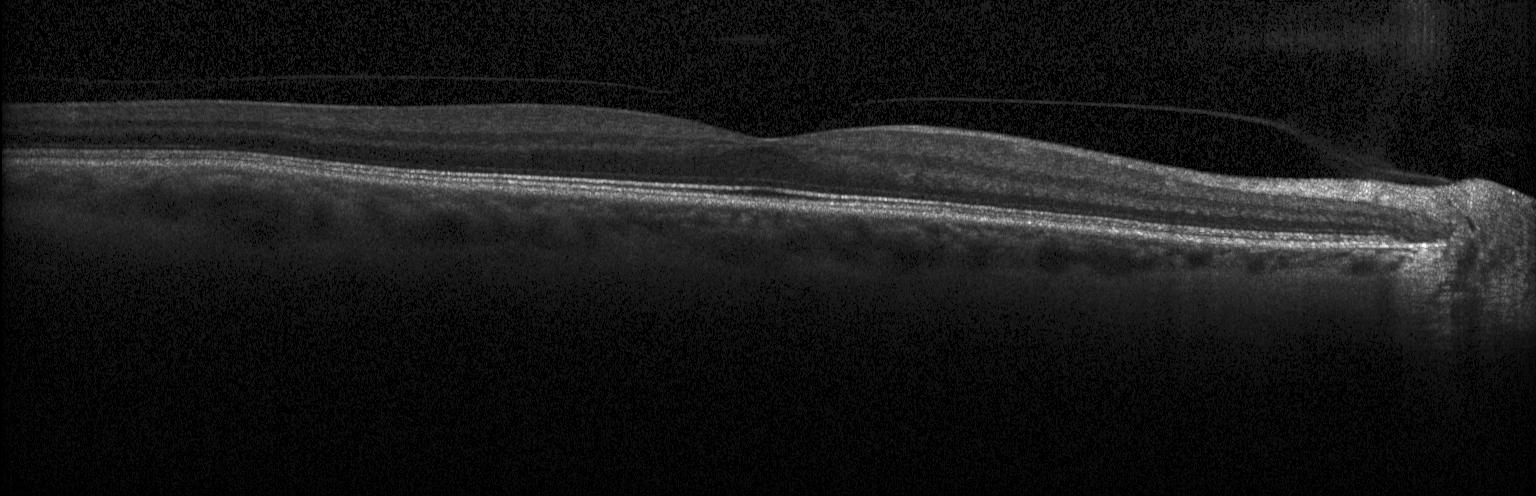 OCT line scan; through the macula; SD-OCT; Heidelberg Spectralis OCT system
Finding: no evidence of choroidal neovascularization, diabetic macular edema, or drusen.